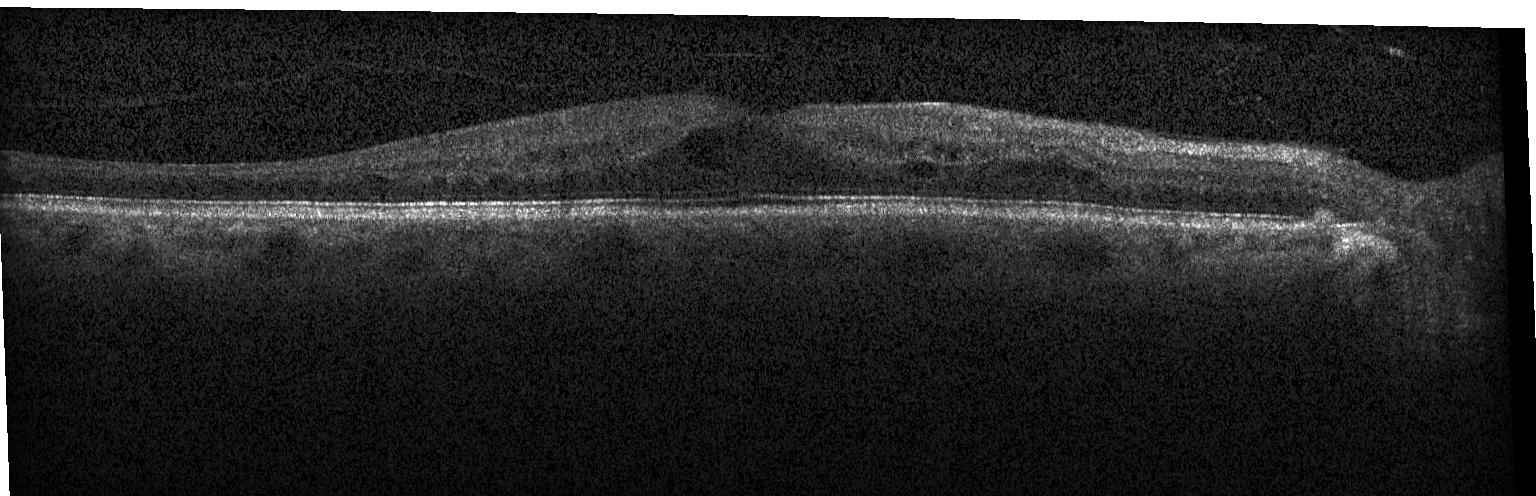 Optical coherence tomography B-scan
Diagnosis: DME.